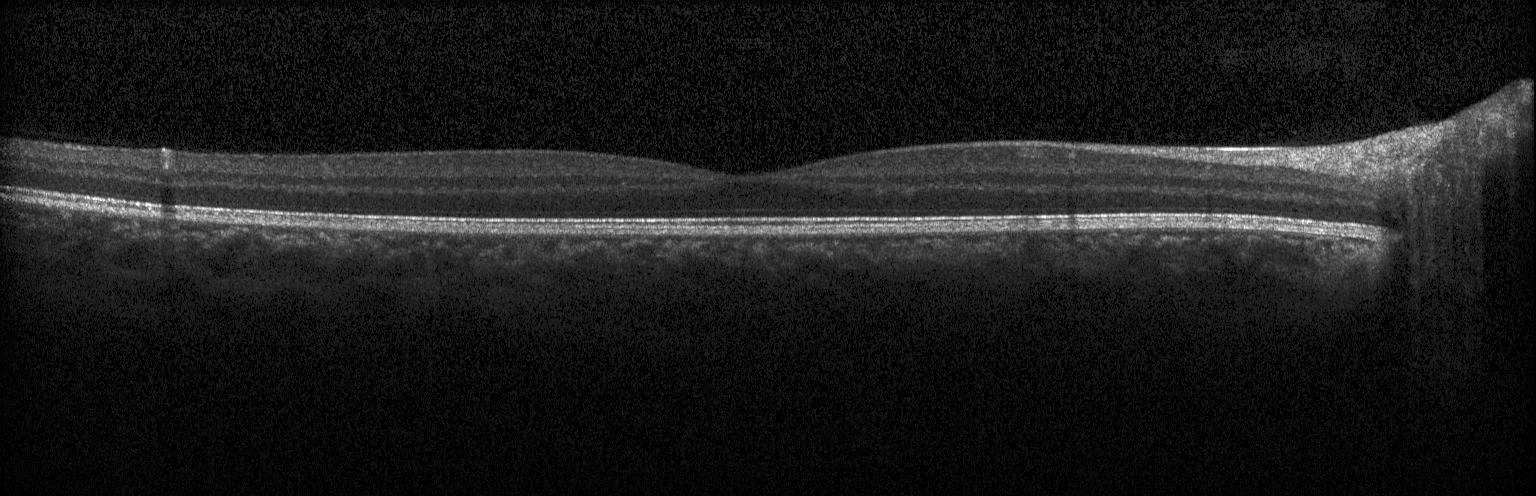
Dx: no choroidal neovascularization, no diabetic macular edema, and no drusen.